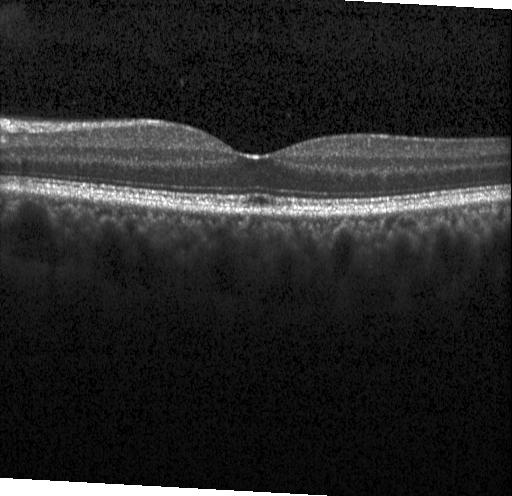
Spectral-domain OCT · optical coherence tomography scan · fovea-centered
Assessment: no evidence of choroidal neovascularization, diabetic macular edema, or drusen.